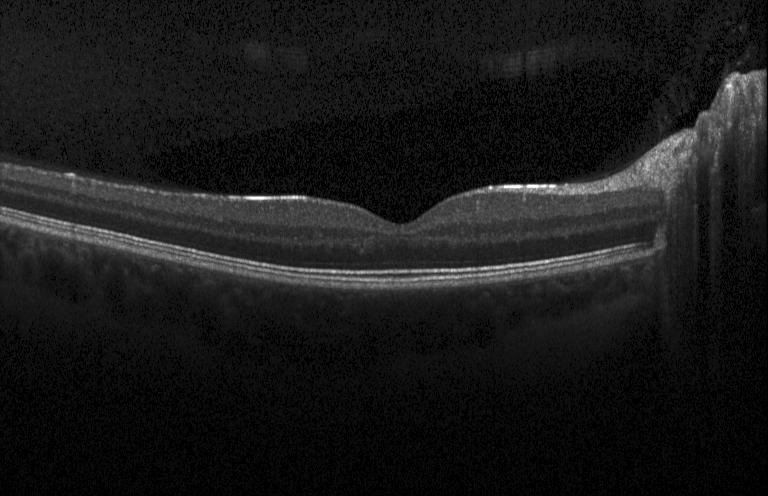

Through the macula, spectral-domain optical coherence tomography, Heidelberg Spectralis OCT system, retinal OCT B-scan. Diagnosis: no CNV, DME, or drusen.